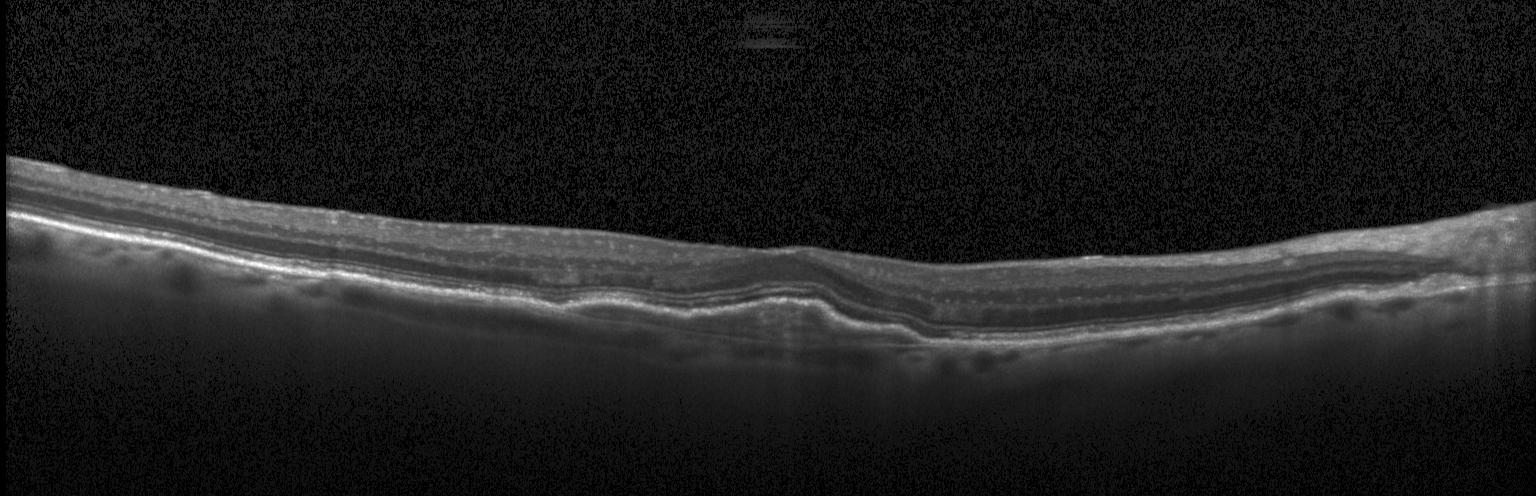
OCT B-scan.
Finding: choroidal neovascularization (CNV).